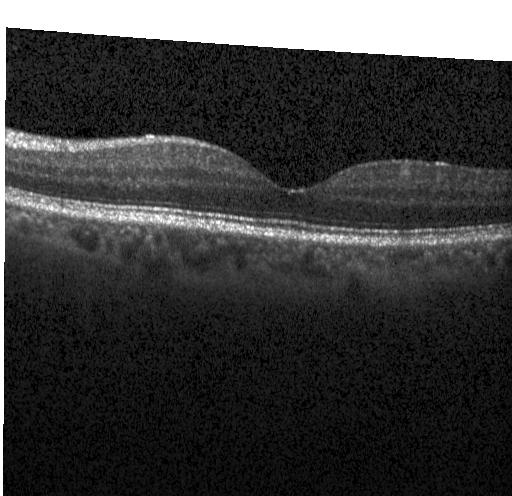

Spectral-domain OCT. Optical coherence tomography scan. Fovea-centered.
Macular OCT: no evidence of choroidal neovascularization, diabetic macular edema, or drusen.